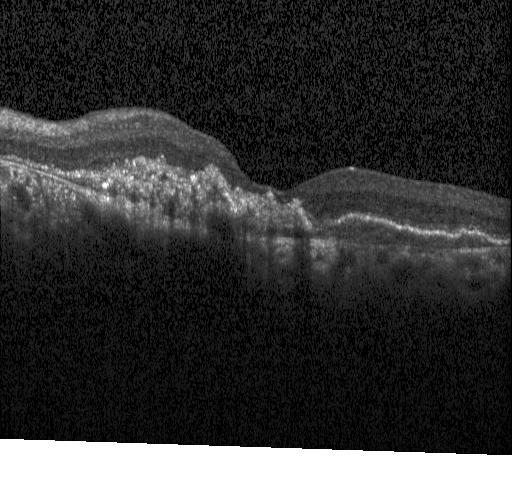 Optical coherence tomography B-scan, fovea-centered, Heidelberg Spectralis OCT system, spectral-domain OCT. Impression: choroidal neovascularization (CNV).